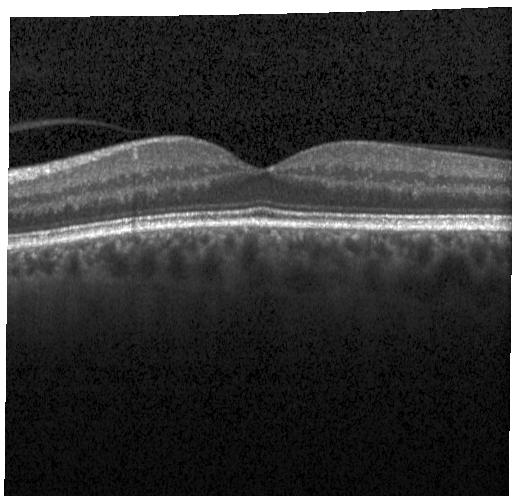

Through the macula. Retinal OCT cross-section
Impression: no choroidal neovascularization, no diabetic macular edema, and no drusen.